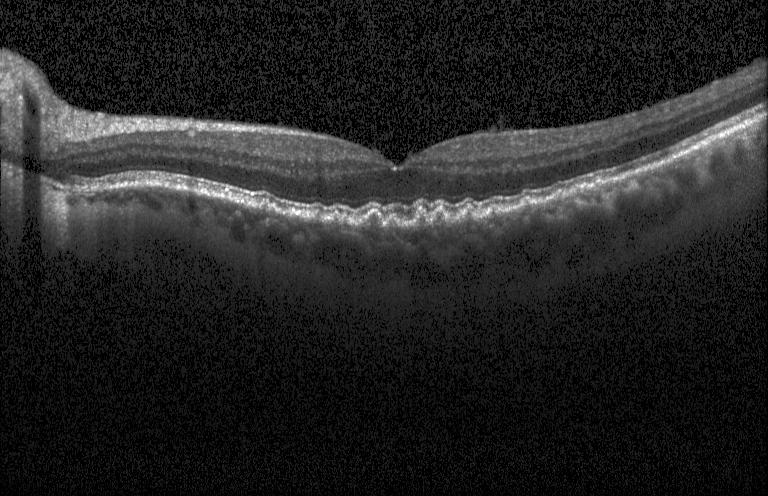
Spectral-domain OCT B-scan: multiple drusen.